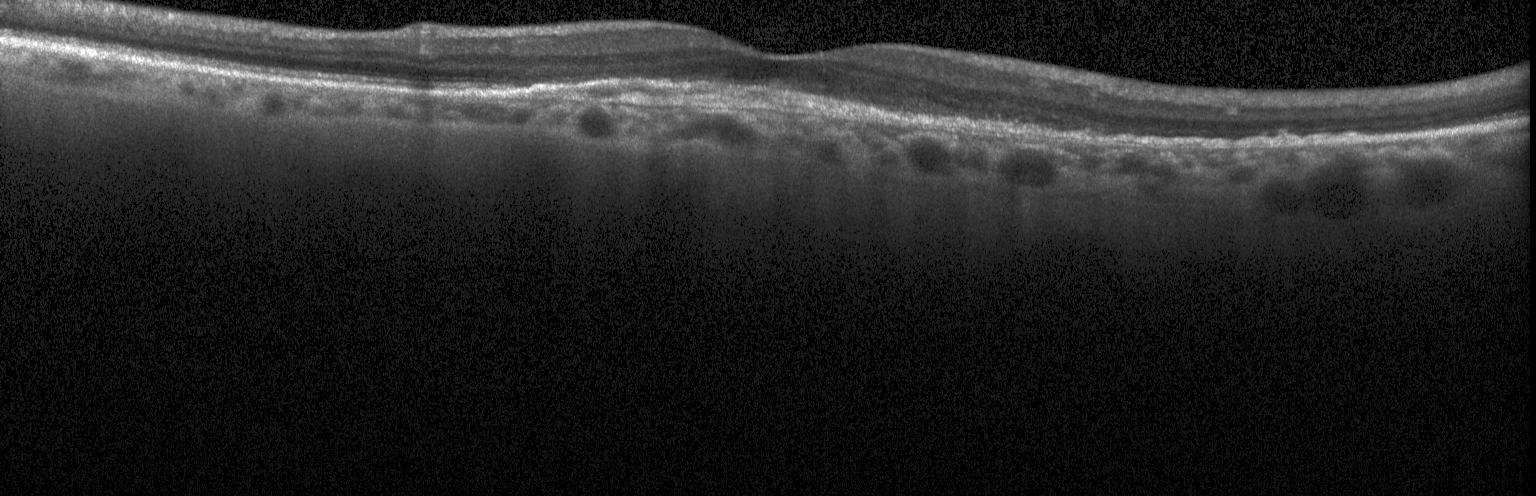
Fovea-centered. OCT B-scan. Spectral-domain OCT. Instrument: Heidelberg Spectralis — Assessment: choroidal neovascularization.